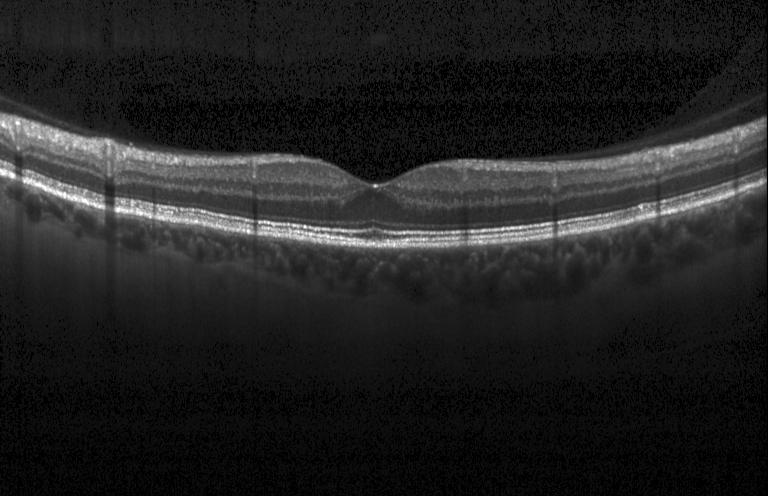 Impression: neither CNV, DME, nor drusen.